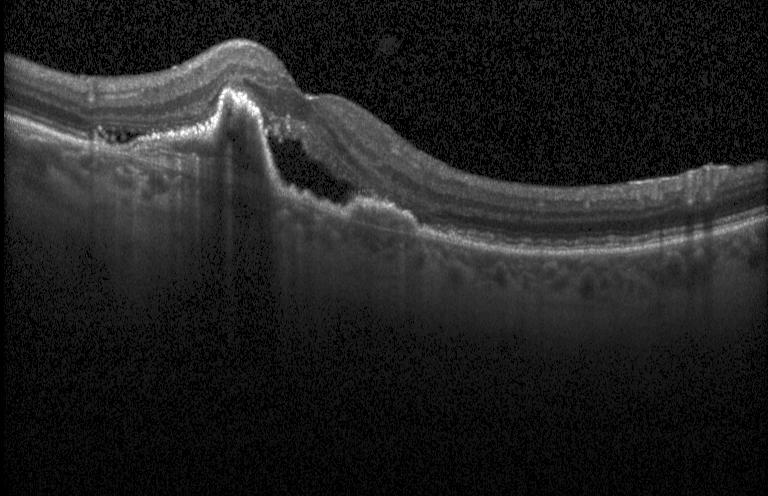 OCT B-scan. Heidelberg Spectralis. Centered on the fovea. Spectral-domain optical coherence tomography. A choroidal neovascular membrane.